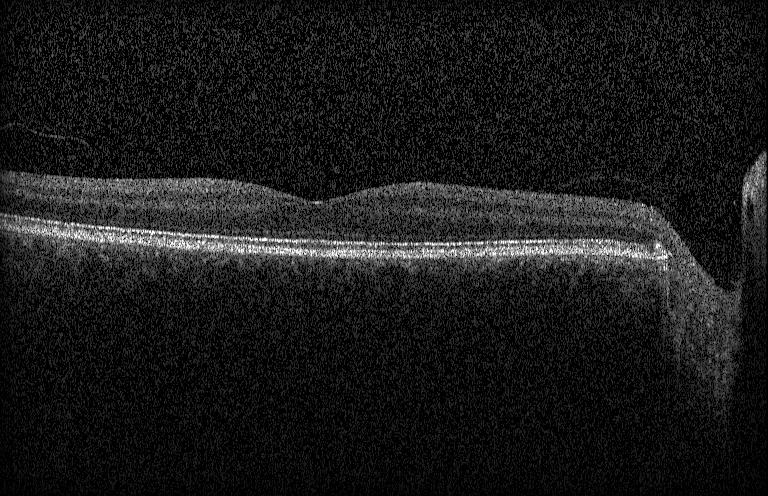

Macular OCT demonstrating no choroidal neovascularization, no diabetic macular edema, and no drusen.